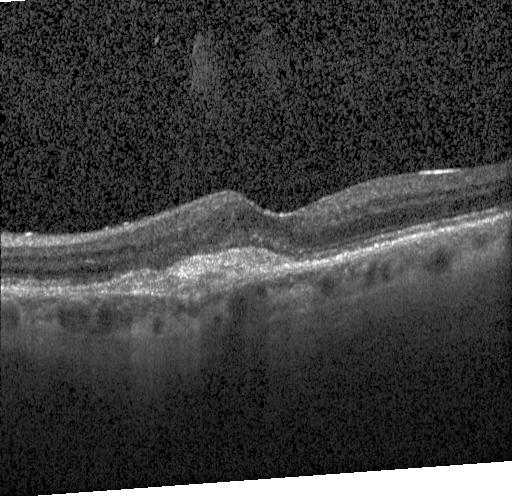
OCT finding: a choroidal neovascular membrane.